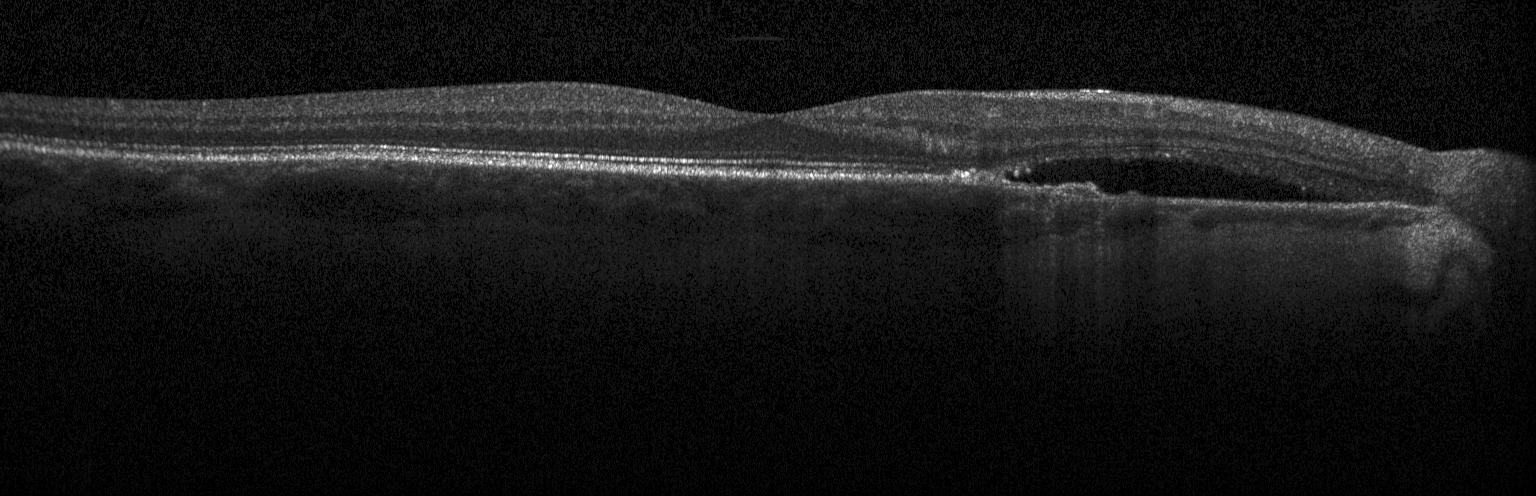 OCT line scan · spectral-domain OCT
This B-scan demonstrates a choroidal neovascular membrane.